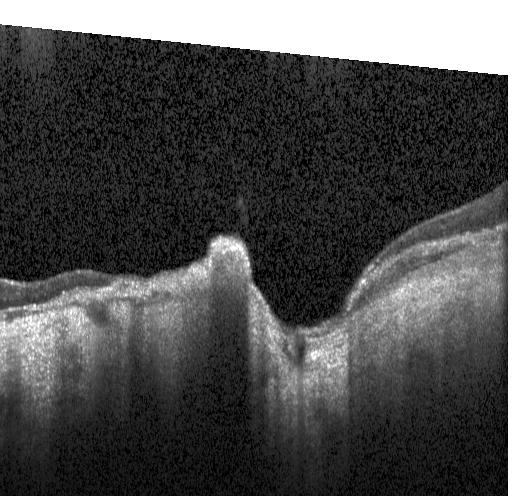 Impression: choroidal neovascularization (CNV).